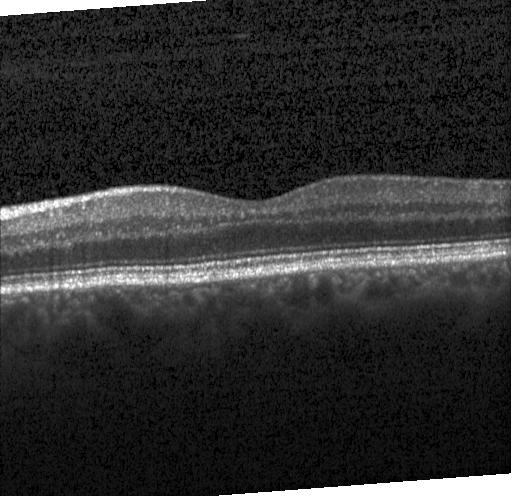
Optical coherence tomography scan. Through the macula. Heidelberg Spectralis OCT system. Spectral-domain optical coherence tomography
No choroidal neovascularization, diabetic macular edema, or drusen.